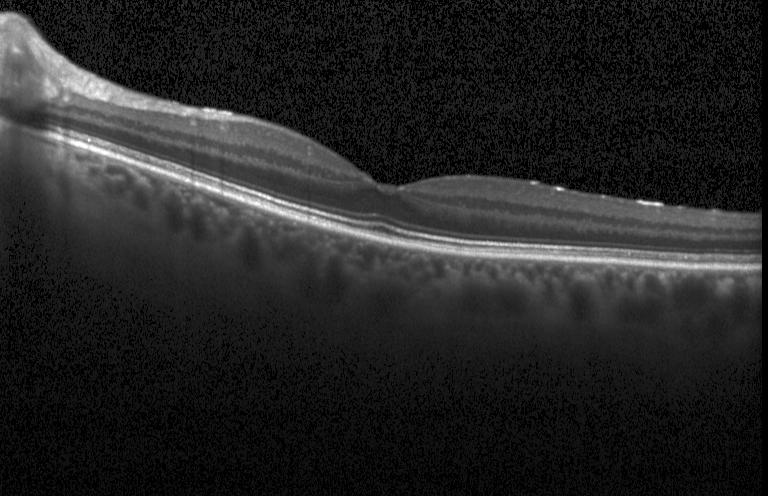

Spectral-domain OCT B-scan: no evidence of choroidal neovascularization, diabetic macular edema, or drusen.